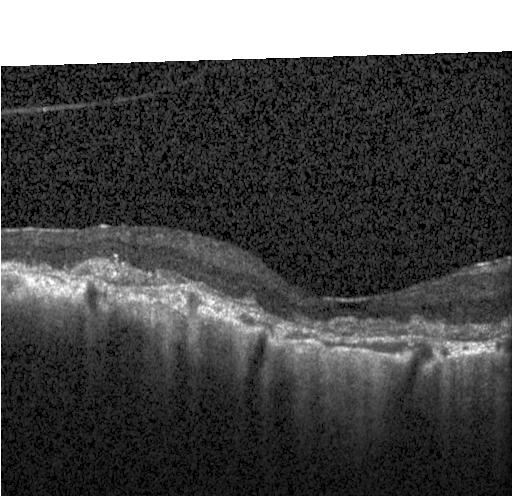

Macular OCT: choroidal neovascularization.